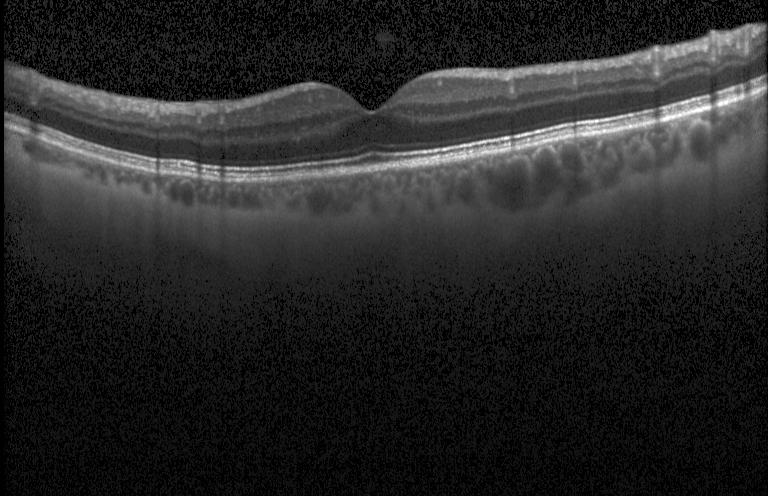

Macular OCT: neither choroidal neovascularization, diabetic macular edema, nor drusen.